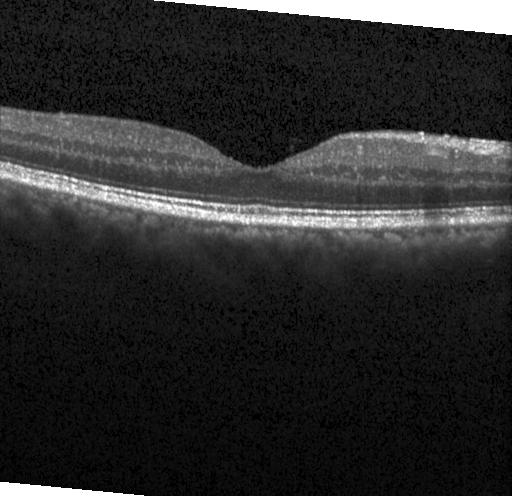 The scan shows no evidence of CNV, DME, or drusen.